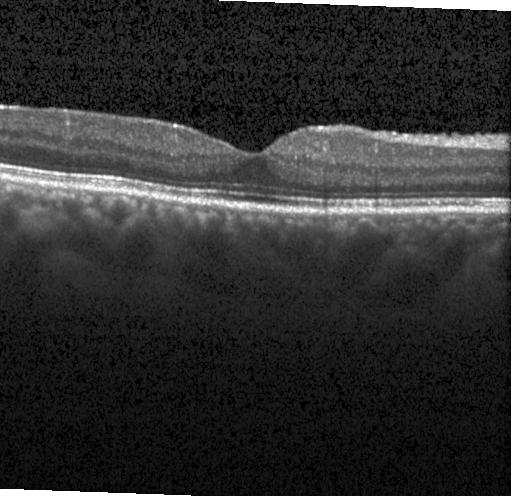 OCT B-scan; centered on the fovea; spectral-domain OCT — Macular OCT: no choroidal neovascularization, diabetic macular edema, or drusen.